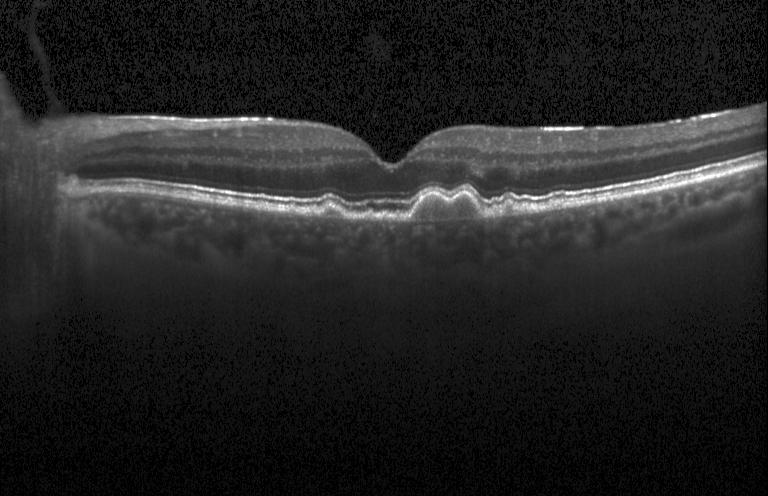 OCT B-scan
Macular OCT: sub-RPE drusenoid deposits.